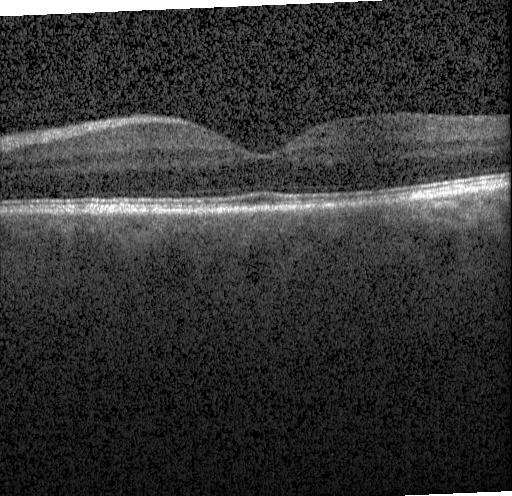

Retinal OCT cross-section
The scan shows no evidence of CNV, DME, or drusen.